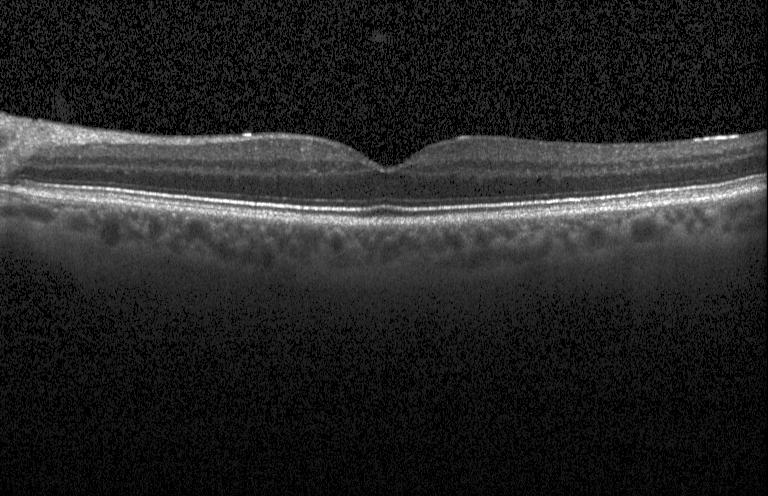
Spectral-domain optical coherence tomography; horizontal scan through the fovea; OCT B-scan. Assessment: no CNV, no DME, and no drusen.